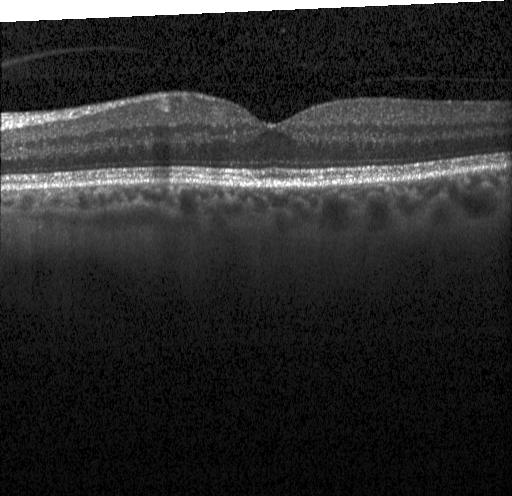 Retinal OCT cross-section · fovea-centered
Finding: no choroidal neovascularization, no diabetic macular edema, and no drusen.